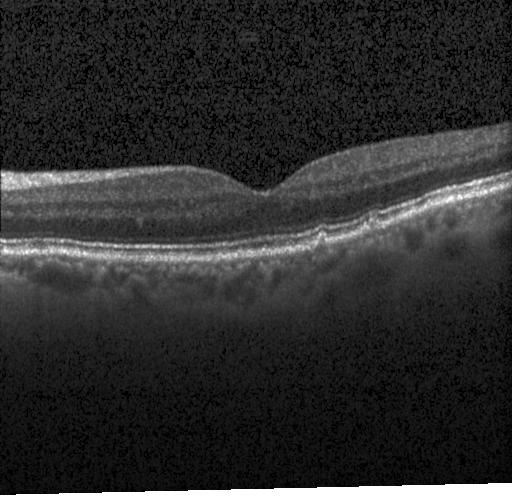

OCT line scan — Impression: multiple drusen.